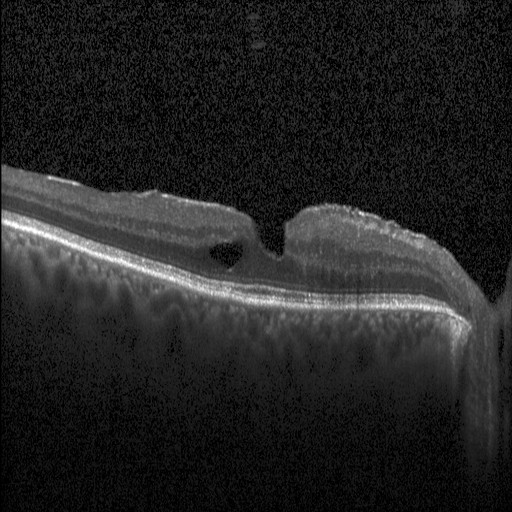
Centered on the fovea. Optical coherence tomography B-scan. SD-OCT. Instrument: Heidelberg Spectralis
DME.